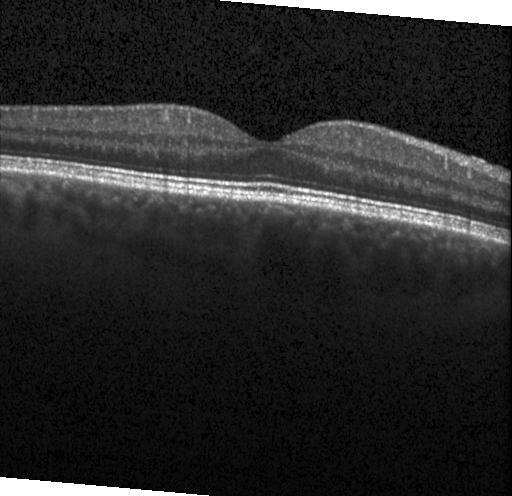
Spectral-domain optical coherence tomography, retinal OCT cross-section, Heidelberg Spectralis. Finding: neither choroidal neovascularization, diabetic macular edema, nor drusen.